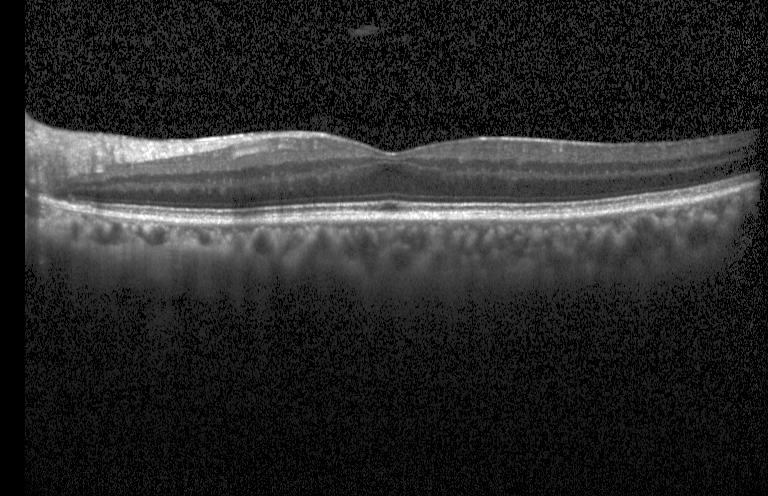
Through the macula · retinal OCT B-scan.
Dx: no choroidal neovascularization, diabetic macular edema, or drusen.